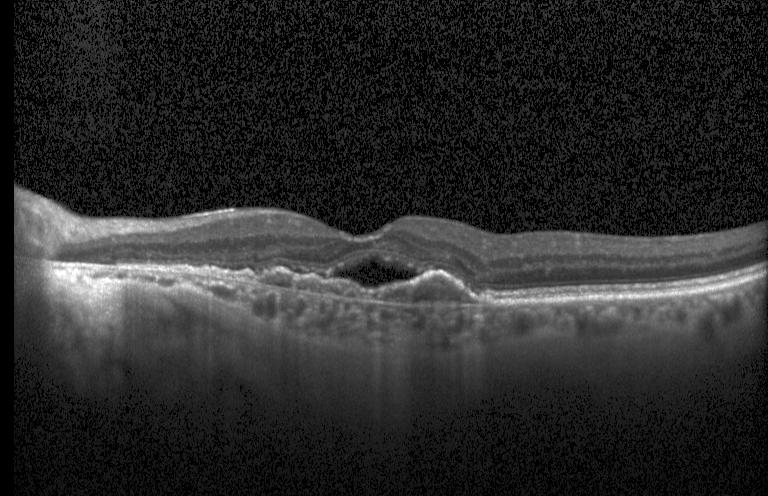 Heidelberg Spectralis. SD-OCT. Retinal OCT cross-section. Fovea-centered. Choroidal neovascularization (CNV).